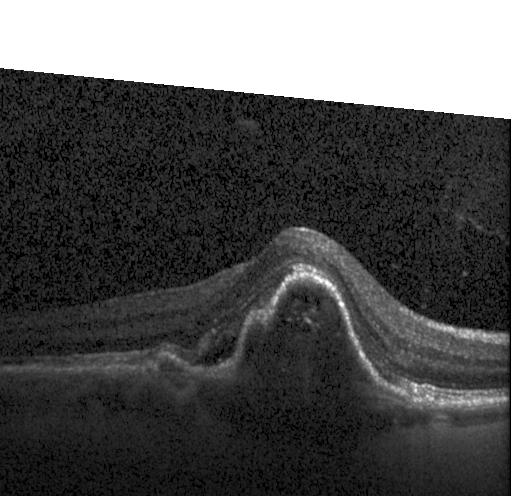
Optical coherence tomography scan — A choroidal neovascular membrane.